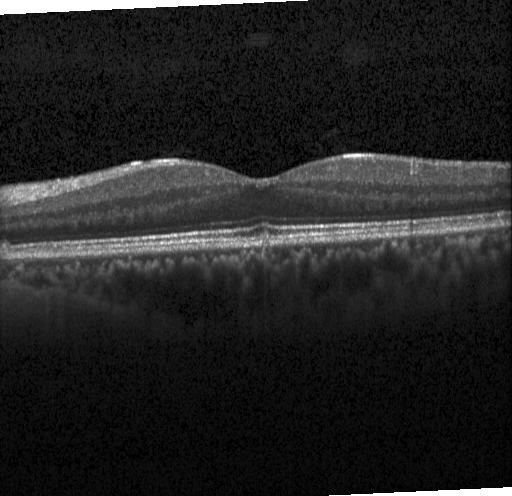

Optical coherence tomography scan. Macular scan — Assessment: no CNV, no DME, and no drusen.